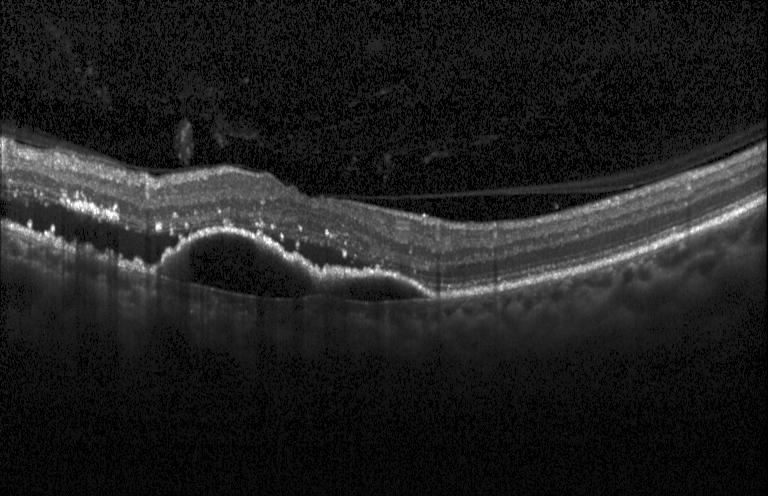
Horizontal scan through the fovea, Heidelberg Spectralis, optical coherence tomography scan.
Macular OCT: a choroidal neovascular membrane.